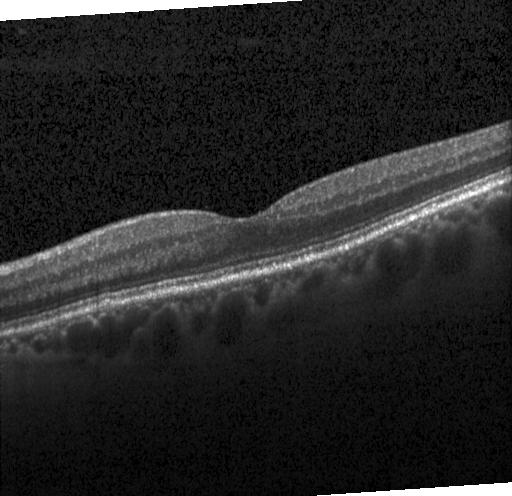
Instrument: Heidelberg Spectralis · OCT line scan · spectral-domain OCT · horizontal scan through the fovea — The scan shows neither CNV, DME, nor drusen.